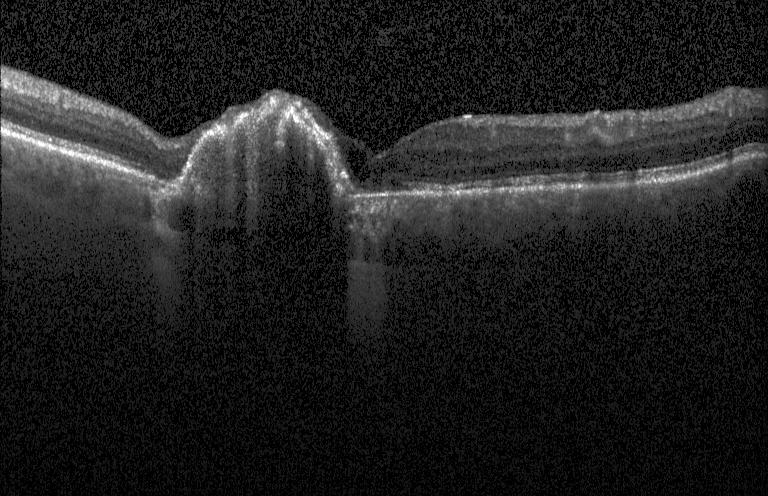

Finding: choroidal neovascularization.